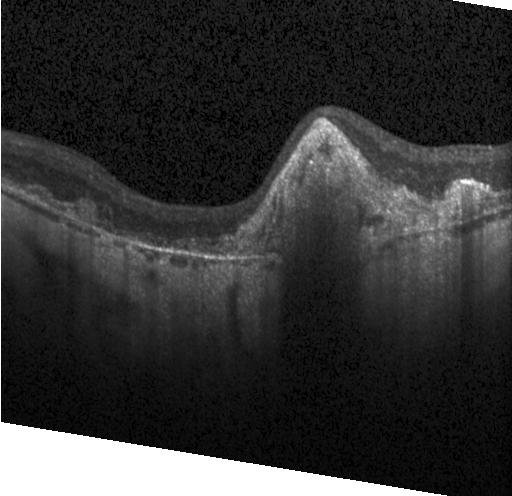
OCT scan showing choroidal neovascularization (CNV).